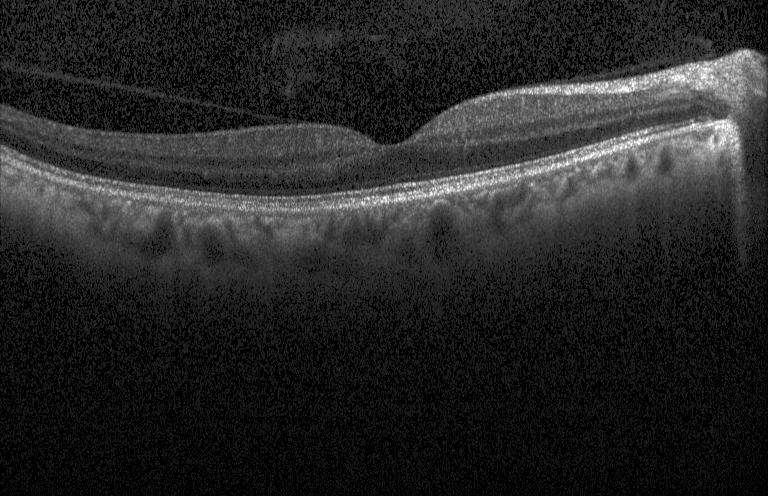 Optical coherence tomography B-scan, instrument: Heidelberg Spectralis.
This B-scan demonstrates no evidence of choroidal neovascularization, diabetic macular edema, or drusen.